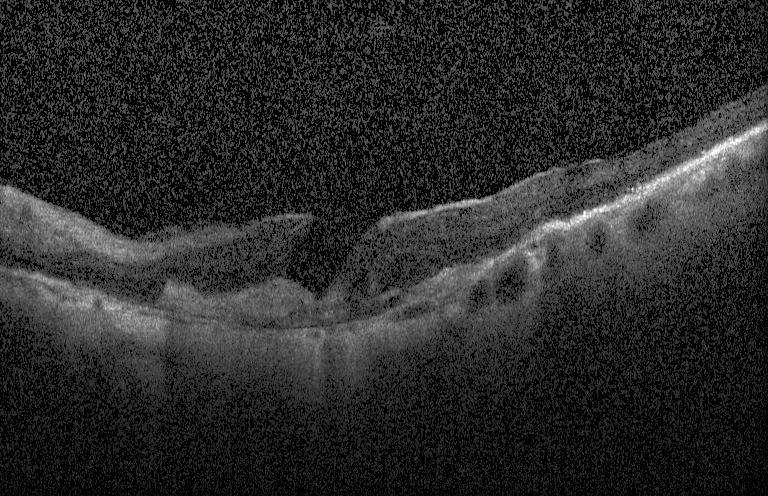

Assessment: a choroidal neovascular membrane.